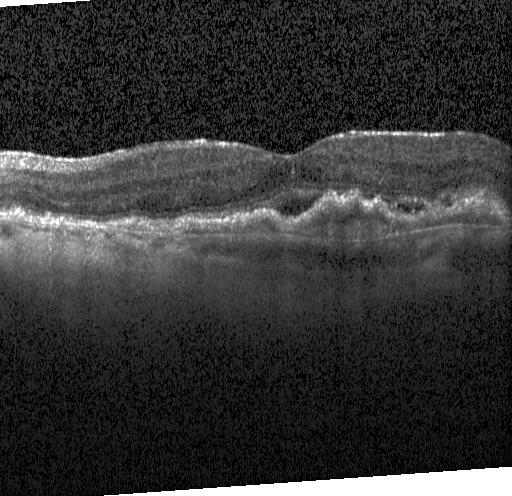
Finding: CNV.